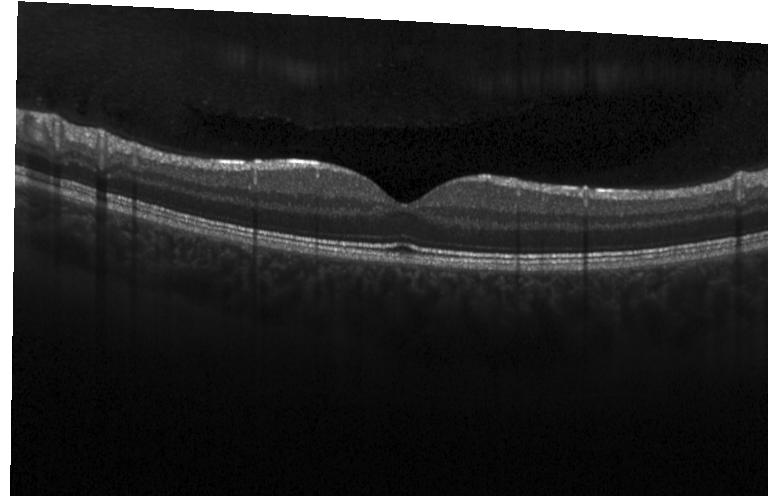
Diagnosis: neither choroidal neovascularization, diabetic macular edema, nor drusen.